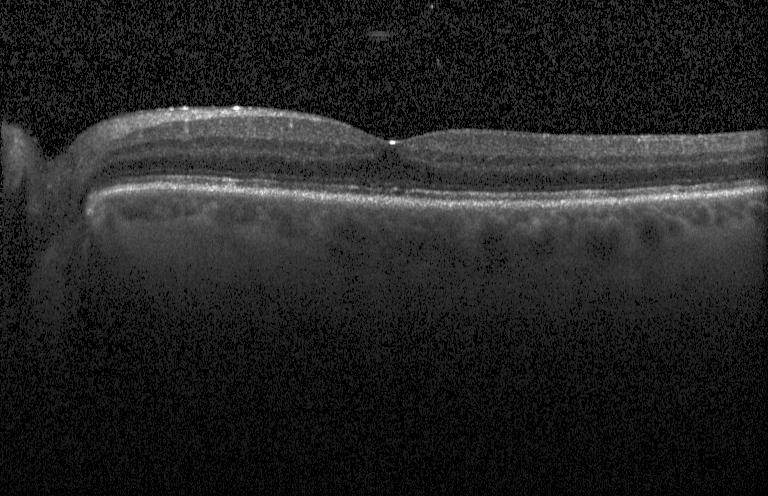

Centered on the fovea. Optical coherence tomography scan. Spectral-domain optical coherence tomography. Heidelberg Spectralis
This B-scan demonstrates no choroidal neovascularization, no diabetic macular edema, and no drusen.